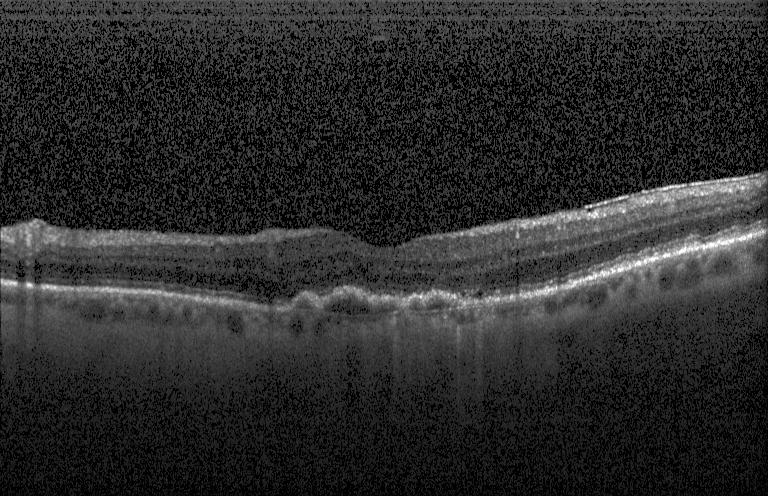 Retinal OCT cross-section. Finding: CNV.